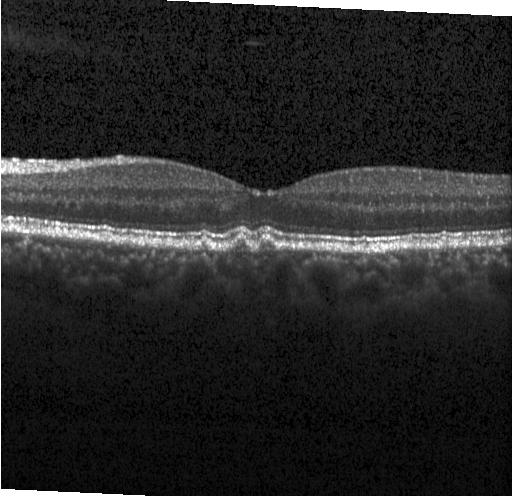 Optical coherence tomography scan · acquired on a Heidelberg Spectralis
Impression: drusen.